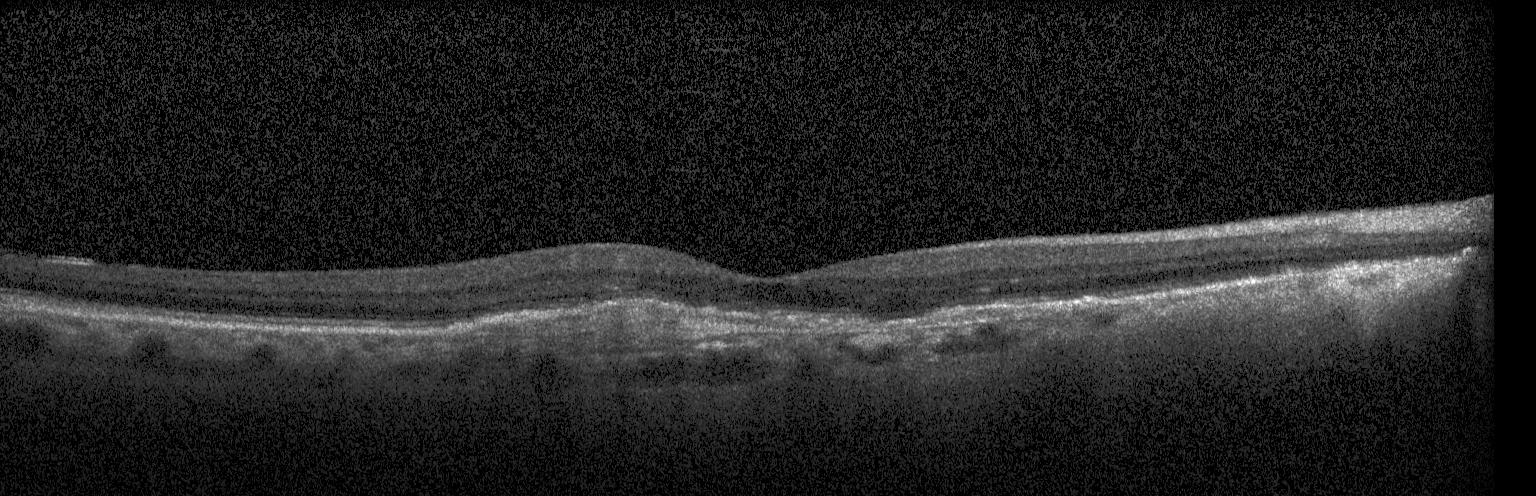

Impression: CNV.